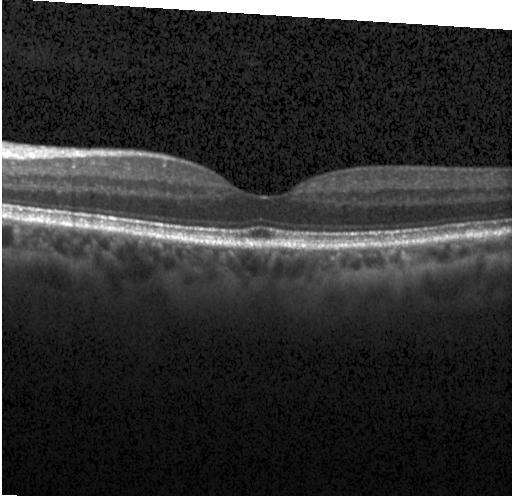

OCT scan showing neither choroidal neovascularization, diabetic macular edema, nor drusen.